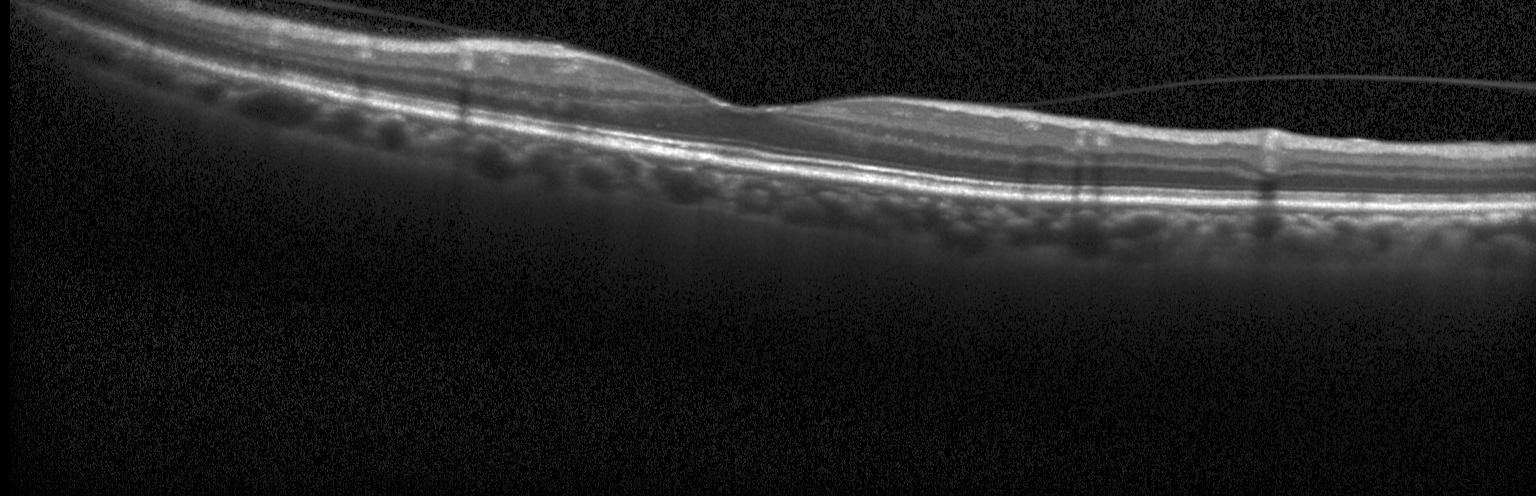

Retinal OCT B-scan; centered on the fovea; spectral-domain optical coherence tomography; Heidelberg Spectralis. Assessment: neither choroidal neovascularization, diabetic macular edema, nor drusen.